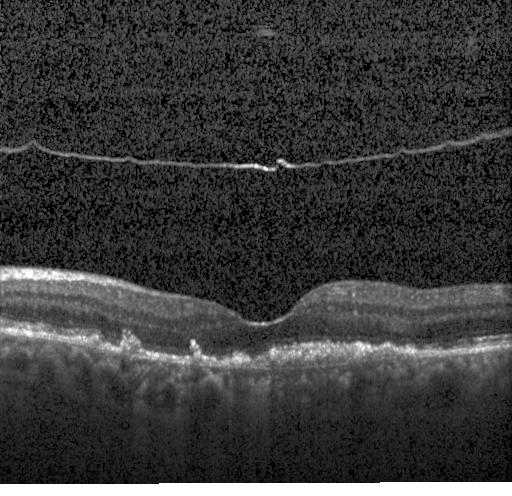

Impression: CNV.